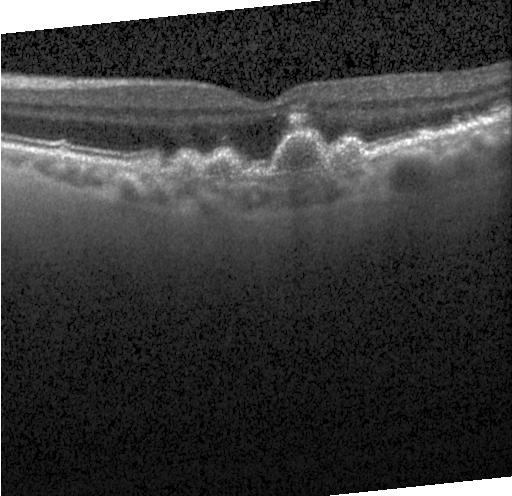 Retinal OCT cross-section · spectral-domain optical coherence tomography · Heidelberg Spectralis · macular scan. Finding: drusen.